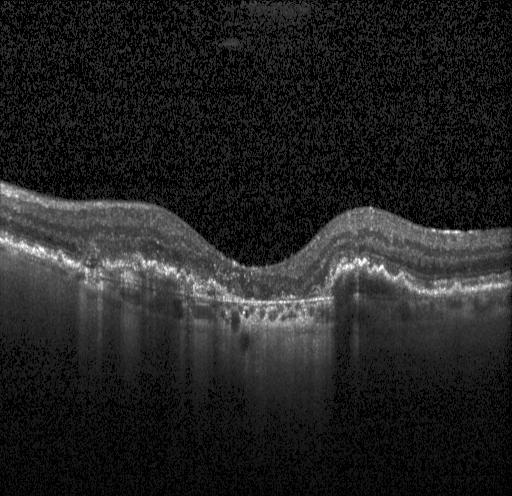
The scan shows a choroidal neovascular membrane.